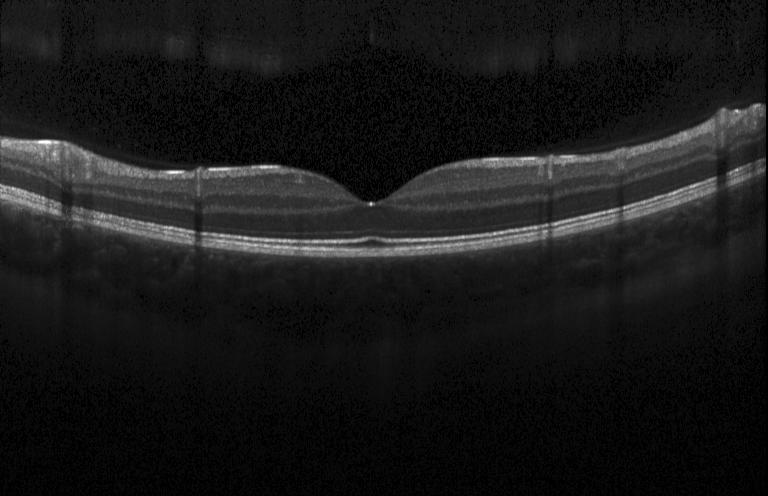 Finding: no CNV, DME, or drusen.